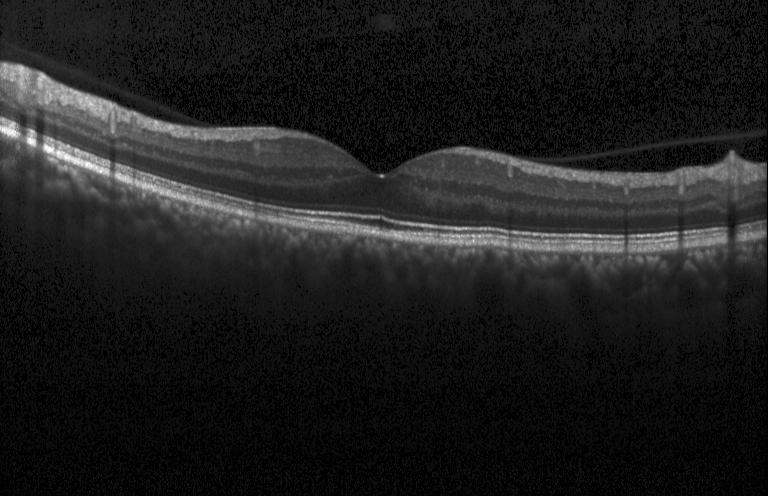

SD-OCT · retinal OCT B-scan. OCT finding: no choroidal neovascularization, no diabetic macular edema, and no drusen.